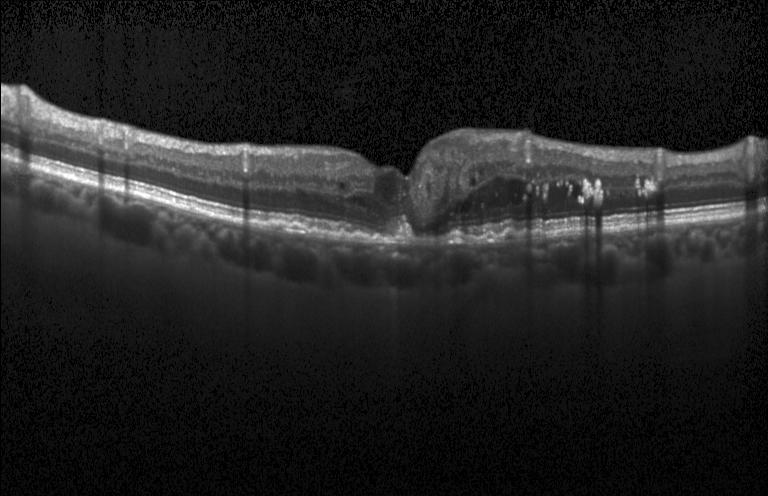

Diagnosis: a choroidal neovascular membrane.